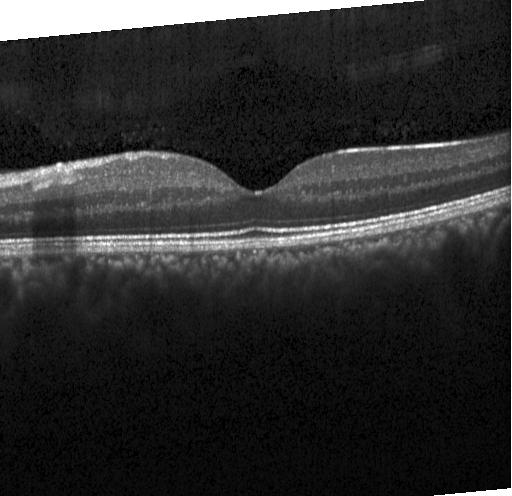 Impression: neither CNV, DME, nor drusen.